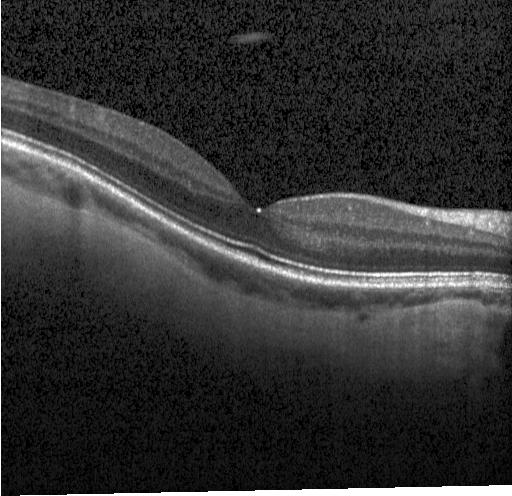
OCT B-scan.
Finding: no evidence of choroidal neovascularization, diabetic macular edema, or drusen.